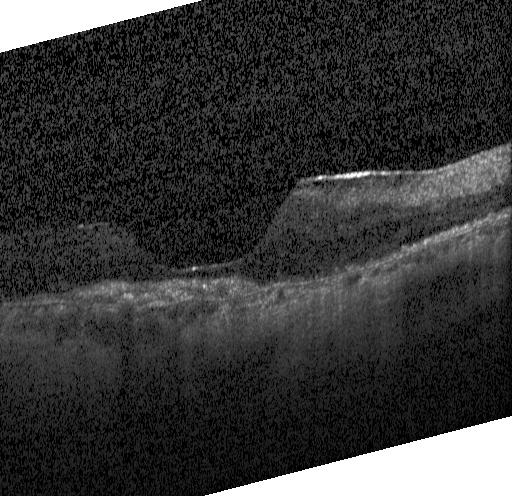 OCT scan showing a choroidal neovascular membrane.